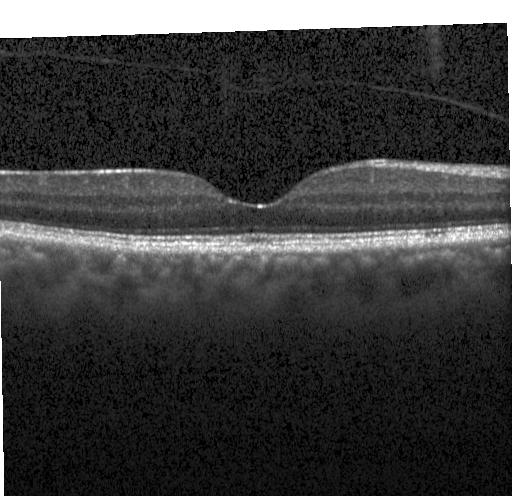
Macular OCT demonstrating no choroidal neovascularization, no diabetic macular edema, and no drusen.